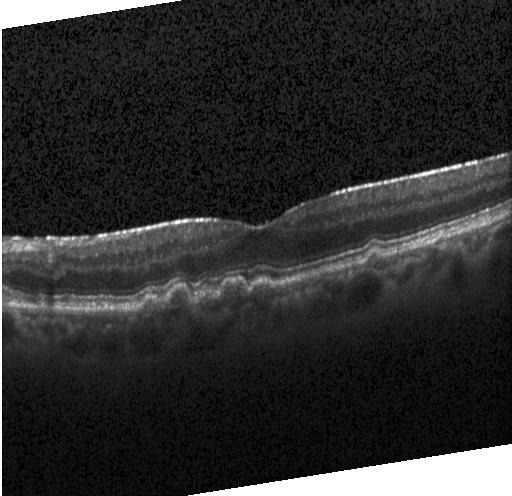

OCT line scan; centered on the fovea.
Sub-RPE drusenoid deposits.